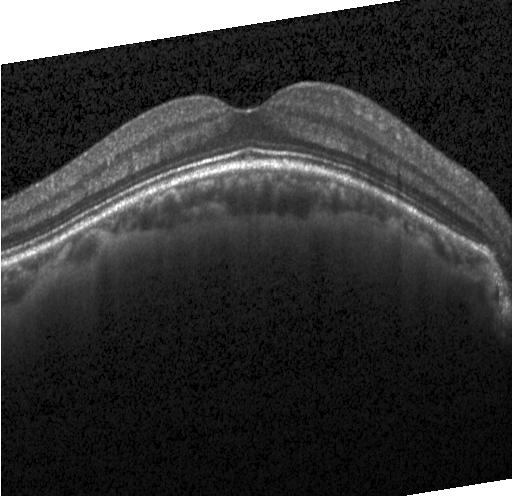
Impression: neither choroidal neovascularization, diabetic macular edema, nor drusen.